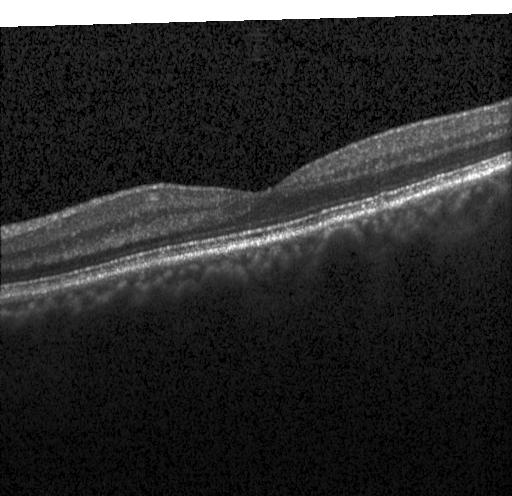 OCT B-scan · fovea-centered — OCT finding: no choroidal neovascularization, no diabetic macular edema, and no drusen.